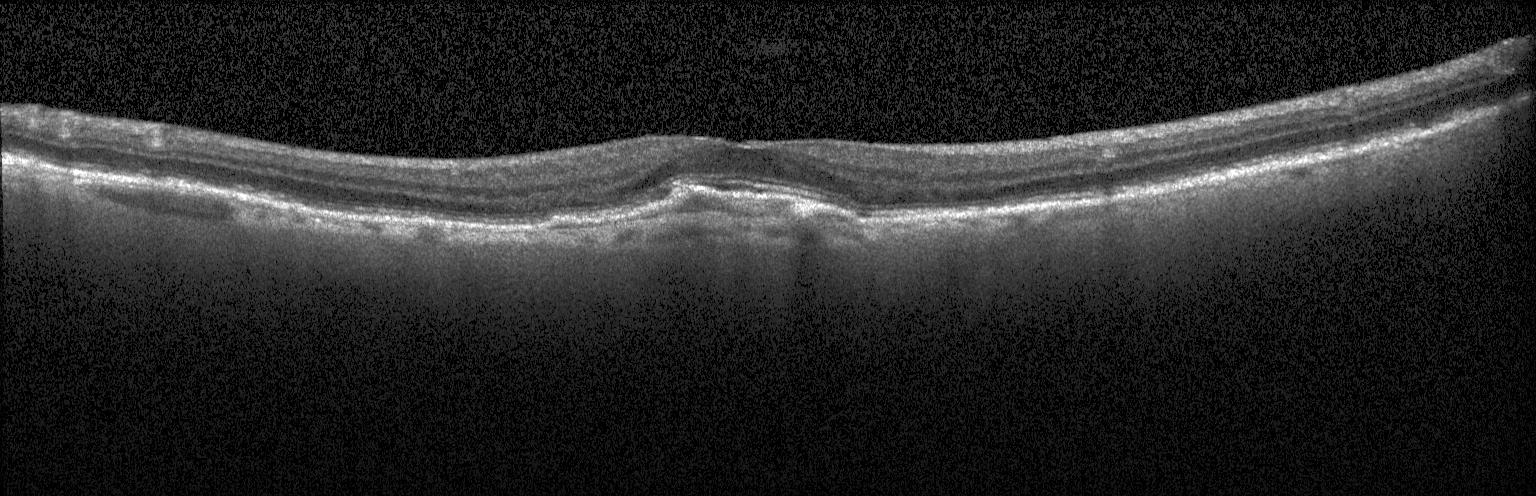 Assessment: a choroidal neovascular membrane.